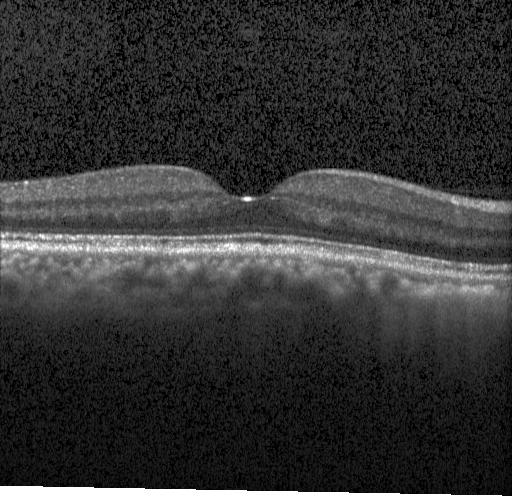 Optical coherence tomography scan
Finding: neither choroidal neovascularization, diabetic macular edema, nor drusen.